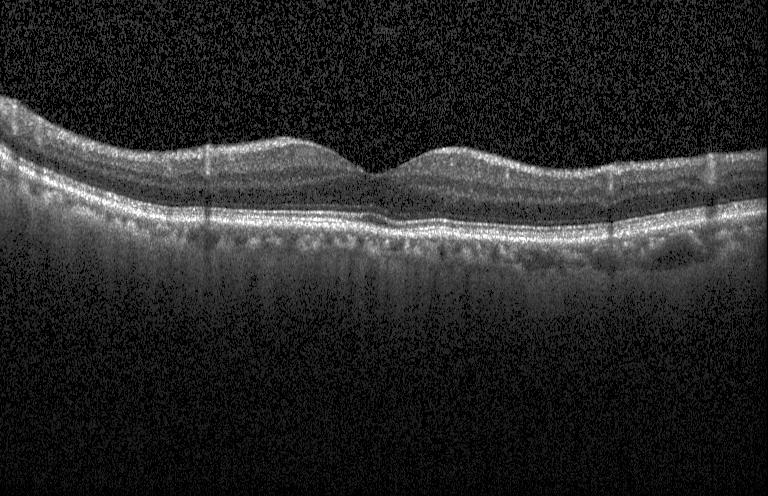

OCT B-scan showing no CNV, DME, or drusen.